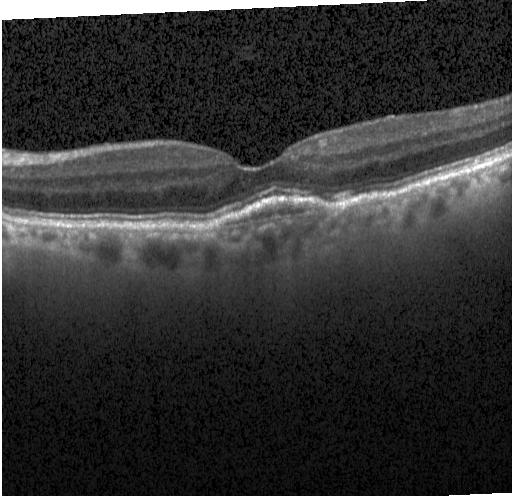 OCT line scan · centered on the fovea. Dx: a choroidal neovascular membrane.